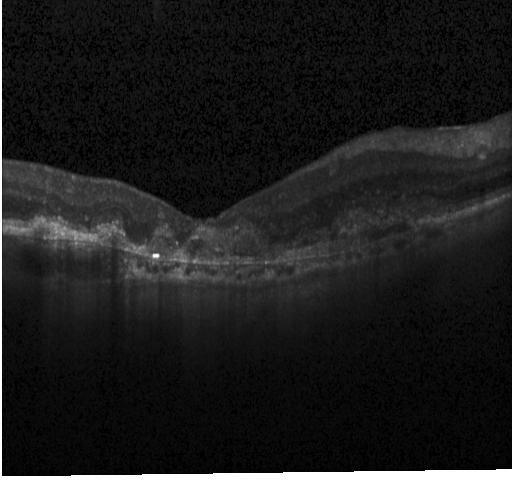

Instrument: Heidelberg Spectralis. SD-OCT. Optical coherence tomography B-scan. Assessment: CNV.